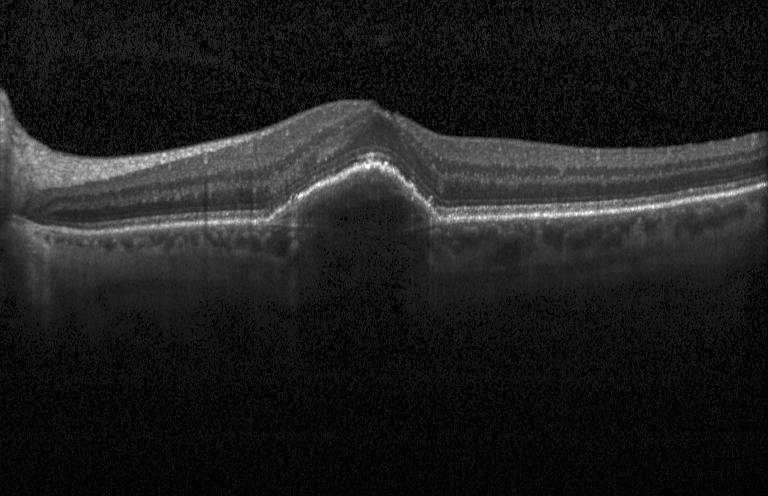
Macular scan; Heidelberg Spectralis OCT system; retinal OCT cross-section; SD-OCT.
Impression: CNV.